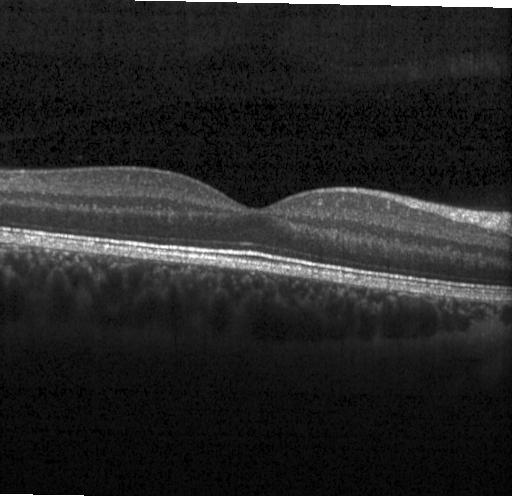
OCT B-scan showing no evidence of choroidal neovascularization, diabetic macular edema, or drusen.